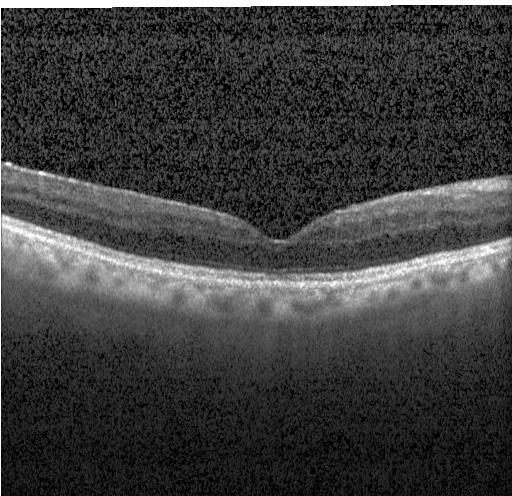

Optical coherence tomography scan
This B-scan demonstrates no evidence of choroidal neovascularization, diabetic macular edema, or drusen.